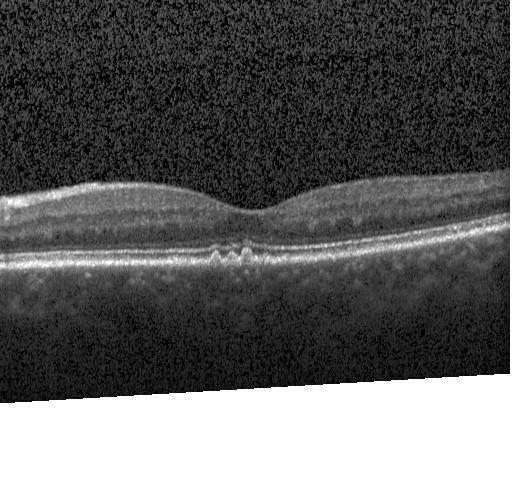 Retinal OCT cross-section showing drusen.